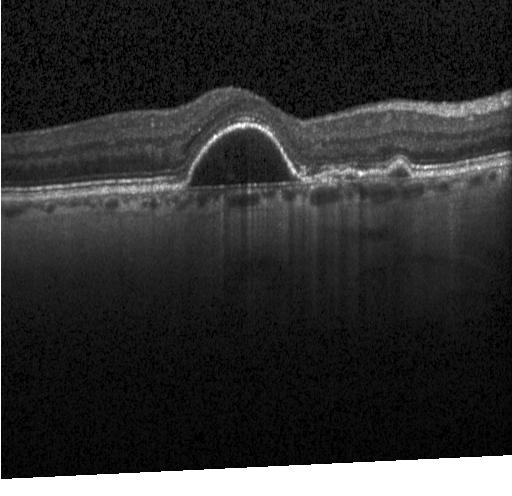

Retinal OCT cross-section showing a choroidal neovascular membrane.